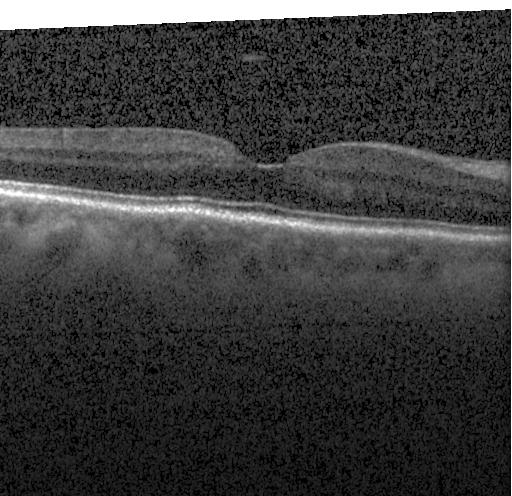

Acquired on a Heidelberg Spectralis. Macular scan. Spectral-domain OCT. Optical coherence tomography scan
Finding: no choroidal neovascularization, no diabetic macular edema, and no drusen.